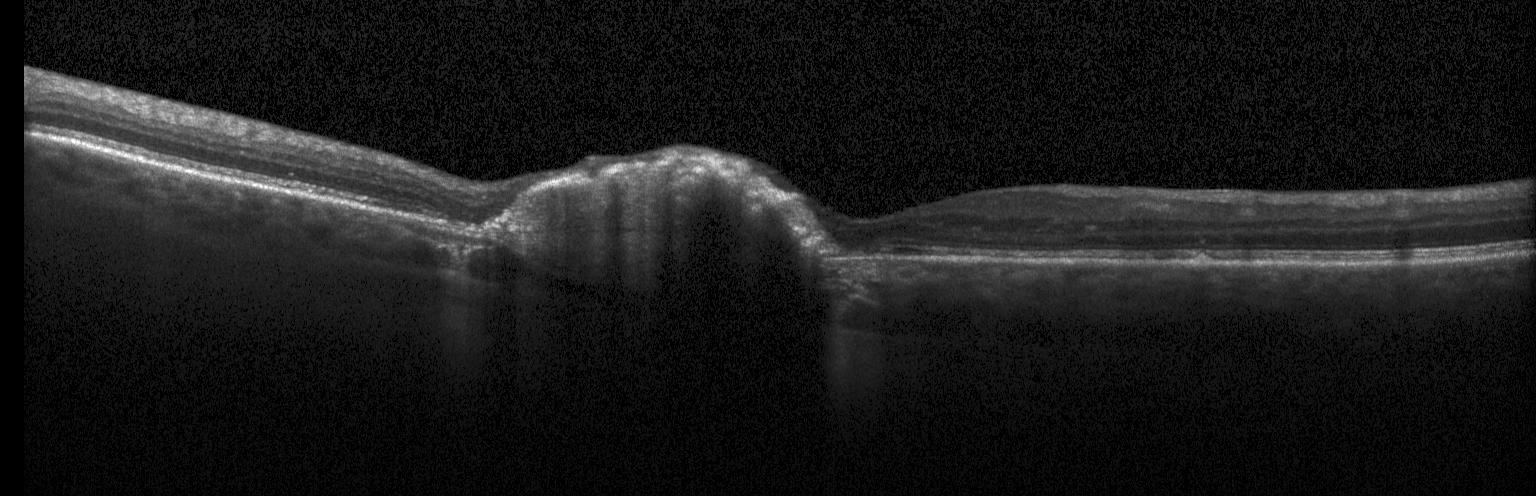

Macular OCT demonstrating choroidal neovascularization (CNV).